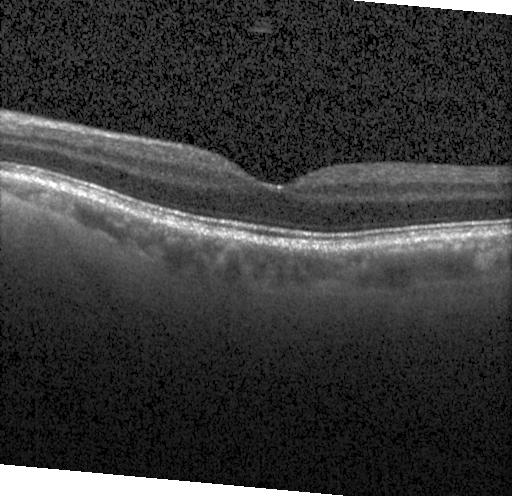 OCT scan showing no choroidal neovascularization, no diabetic macular edema, and no drusen.